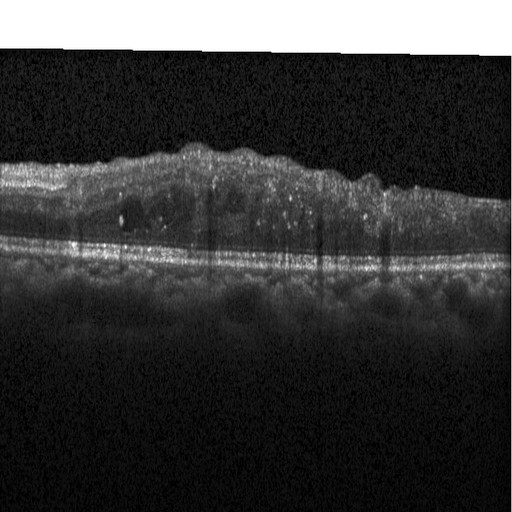
OCT finding: diabetic macular edema (DME).